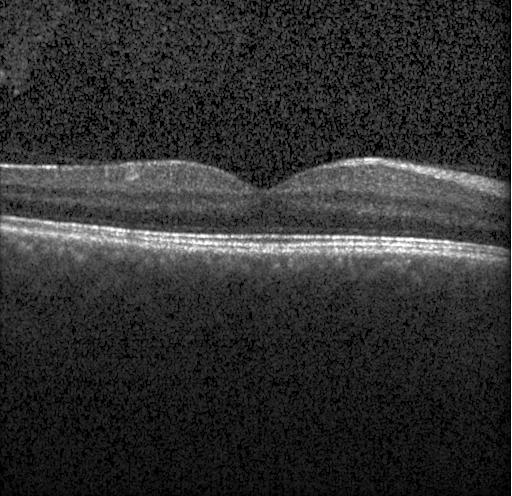 Macular OCT: neither CNV, DME, nor drusen.